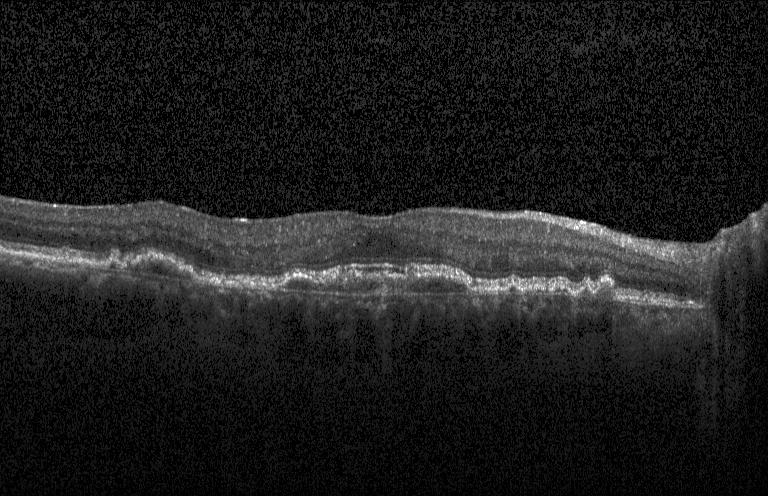

Spectral-domain OCT · Heidelberg Spectralis OCT system · optical coherence tomography B-scan.
A choroidal neovascular membrane.